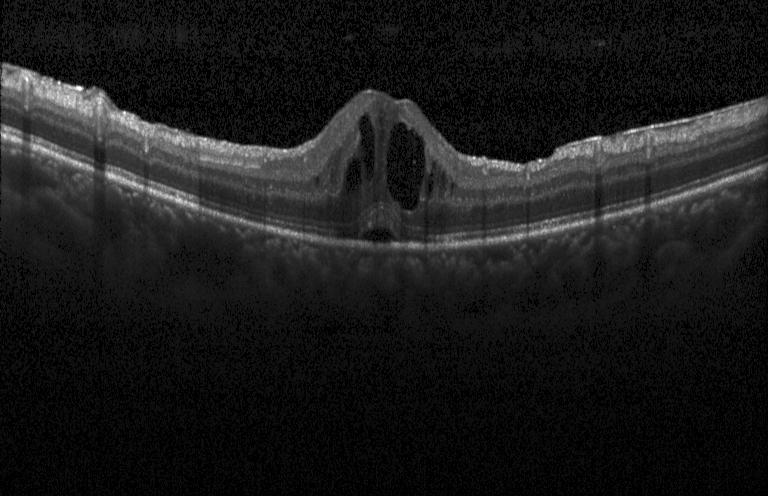

OCT line scan. Spectral-domain optical coherence tomography. Heidelberg Spectralis OCT system. Dx: diabetic macular edema (DME).